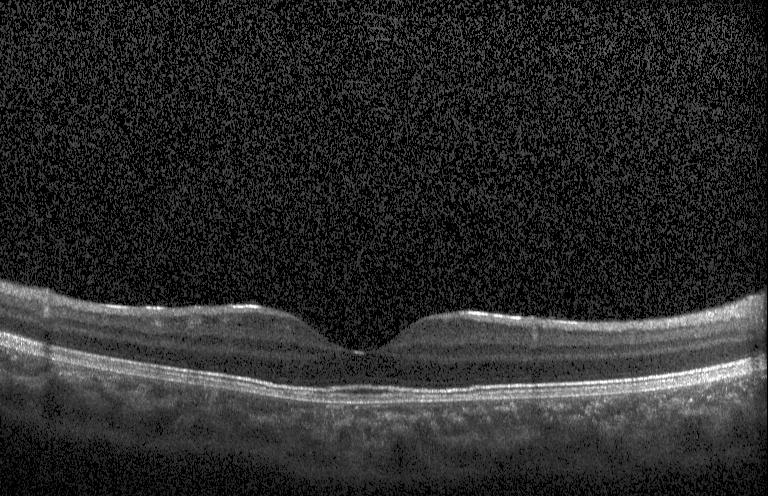
Through the macula, retinal OCT cross-section.
Diagnosis: no CNV, no DME, and no drusen.